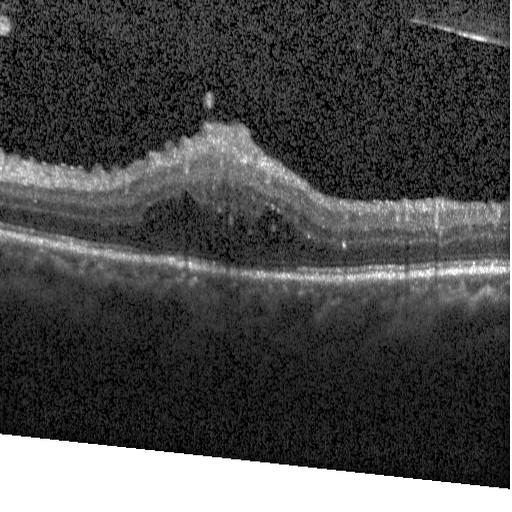
OCT B-scan, fovea-centered, Heidelberg Spectralis, spectral-domain optical coherence tomography.
Assessment: DME.